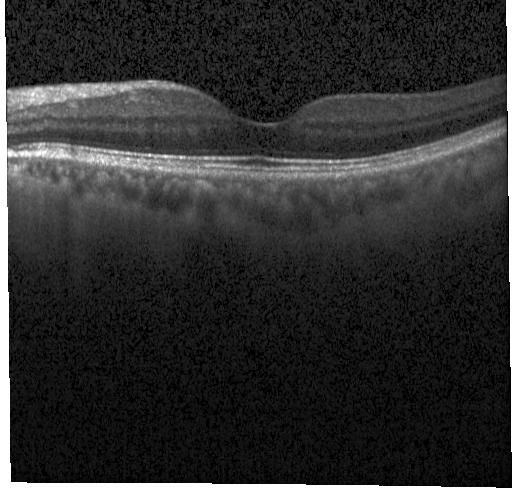 OCT B-scan showing no choroidal neovascularization, no diabetic macular edema, and no drusen.